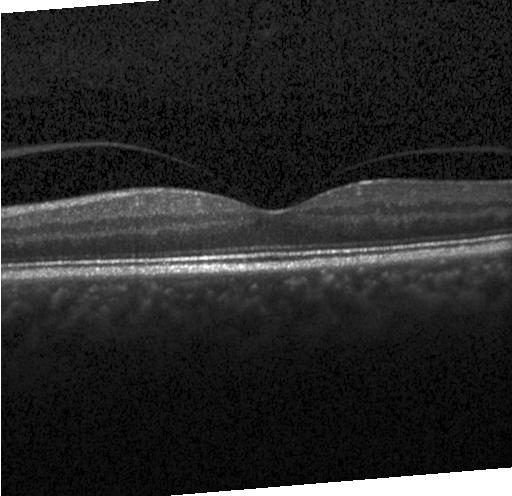
Retinal OCT B-scan
Finding: no choroidal neovascularization, no diabetic macular edema, and no drusen.